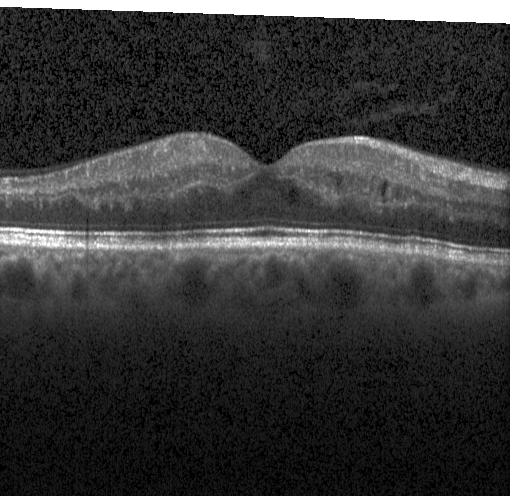

Finding: diabetic macular edema (DME).